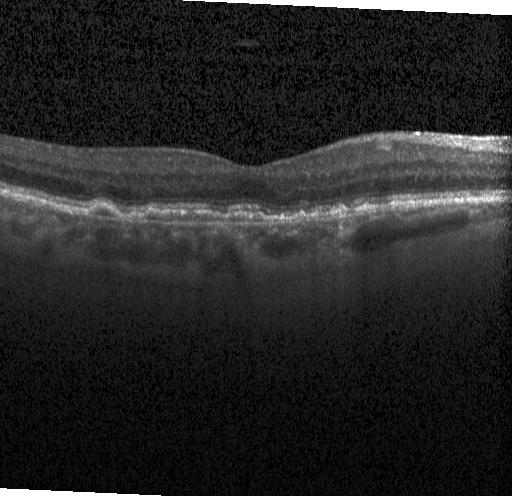
Optical coherence tomography B-scan — This B-scan demonstrates choroidal neovascularization.